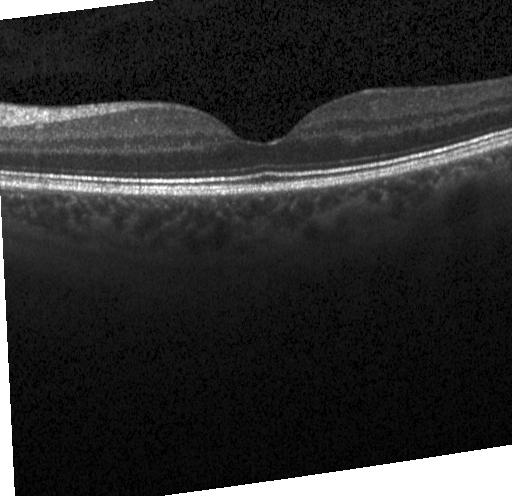 Optical coherence tomography scan; spectral-domain OCT; horizontal scan through the fovea. Diagnosis: no CNV, DME, or drusen.